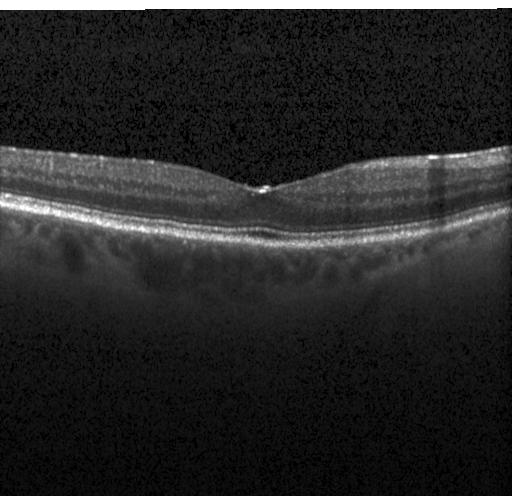
Optical coherence tomography scan. Acquired on a Heidelberg Spectralis. Fovea-centered
Neither CNV, DME, nor drusen.